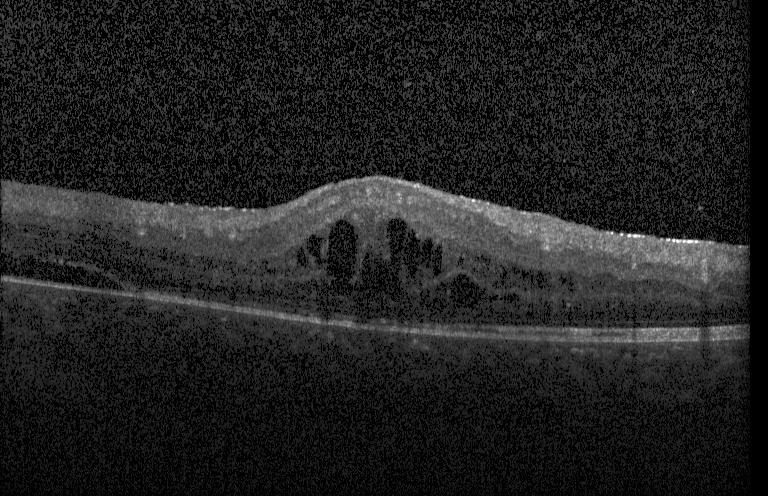 Finding: diabetic macular edema (DME).